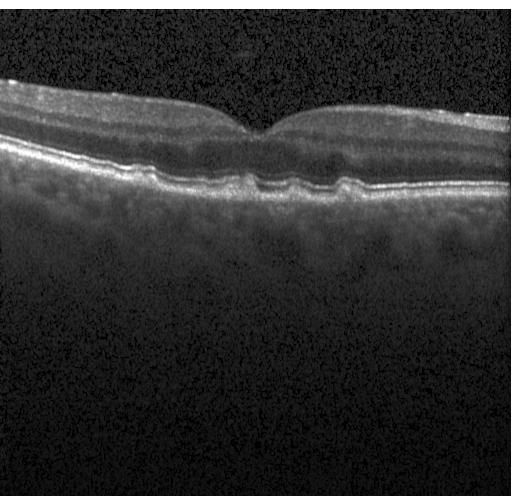
Macular OCT: multiple drusen.